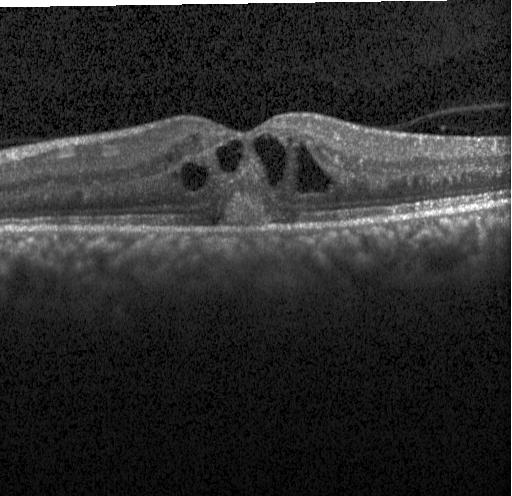

Optical coherence tomography scan · fovea-centered · SD-OCT
OCT finding: choroidal neovascularization.